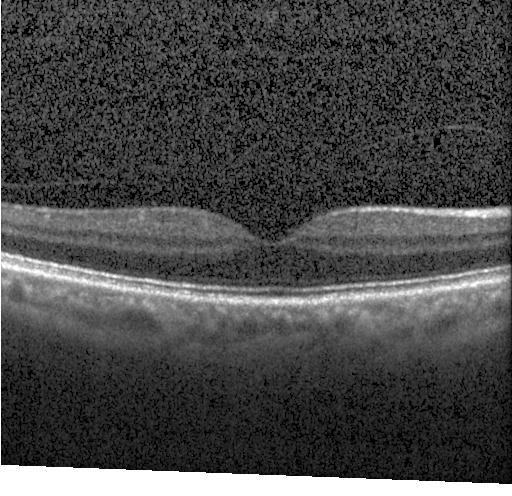
Retinal OCT cross-section — Dx: no evidence of CNV, DME, or drusen.